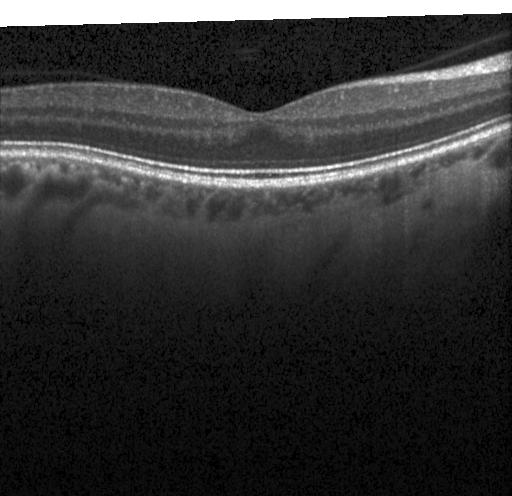
Retinal OCT cross-section showing no choroidal neovascularization, no diabetic macular edema, and no drusen.